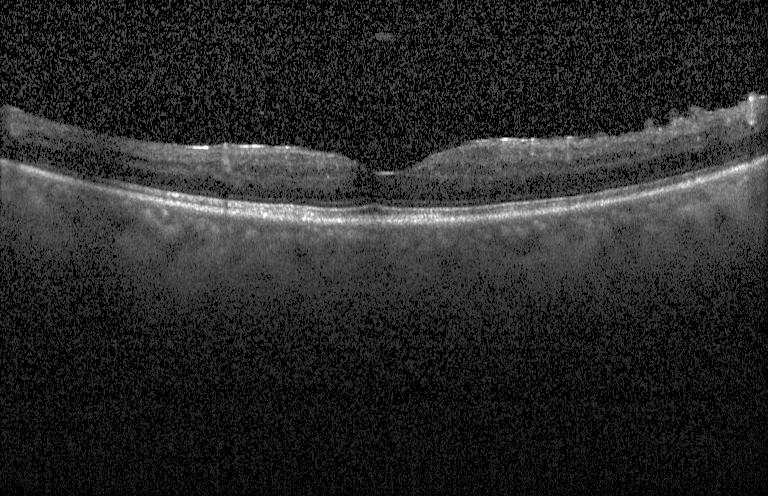 Through the macula · optical coherence tomography scan.
Diagnosis: no CNV, no DME, and no drusen.